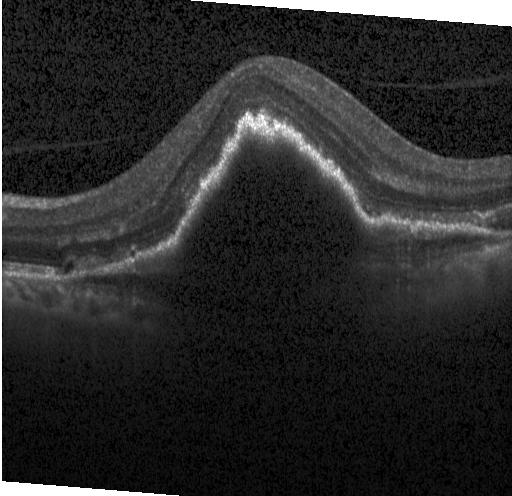
Acquired on a Heidelberg Spectralis. OCT line scan. Diagnosis: a choroidal neovascular membrane.